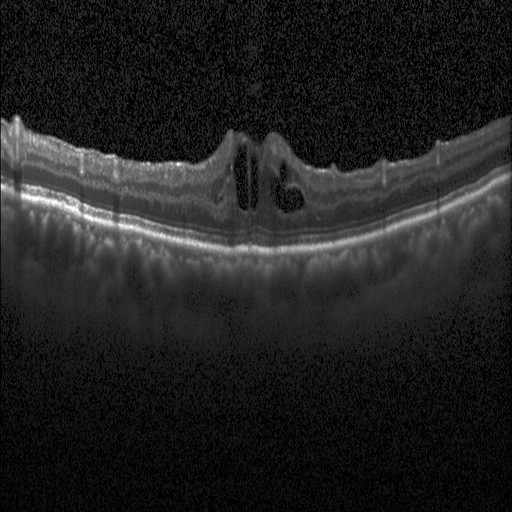 Retinal OCT cross-section. Fovea-centered
Impression: diabetic macular edema.